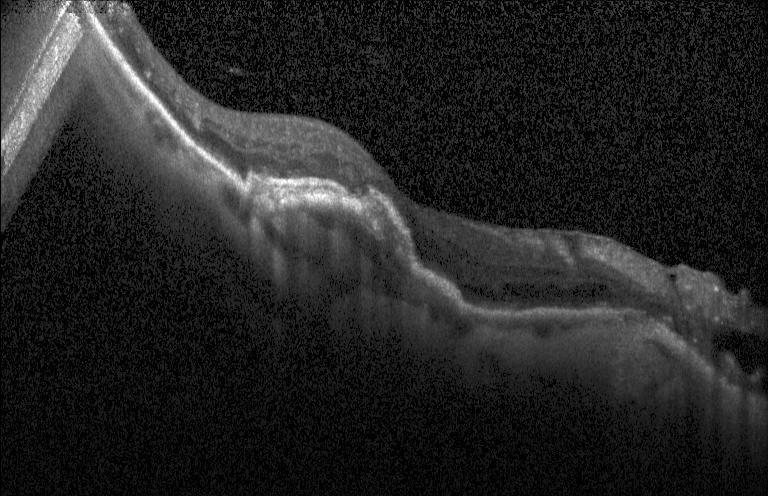 OCT scan showing choroidal neovascularization.